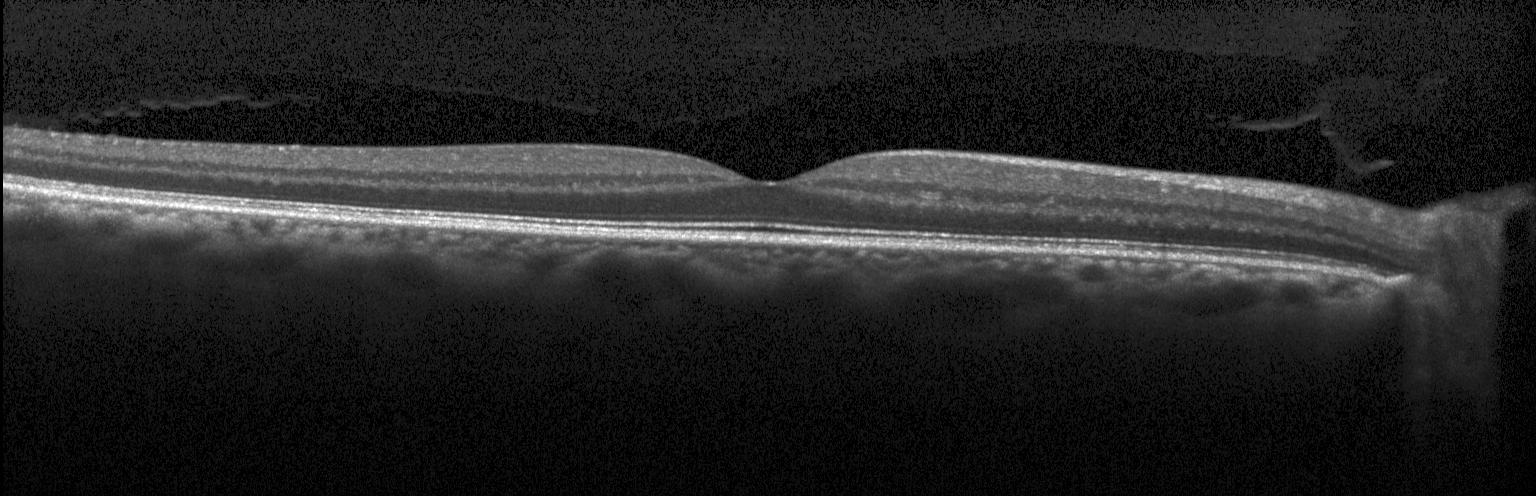 Macular scan; OCT B-scan; Heidelberg Spectralis OCT system; spectral-domain OCT
Finding: neither CNV, DME, nor drusen.